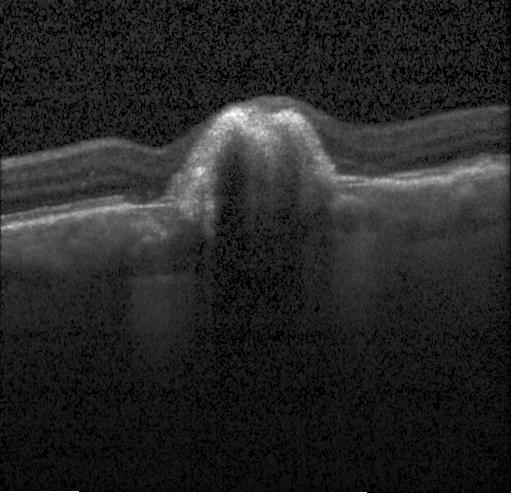 OCT B-scan showing a choroidal neovascular membrane.